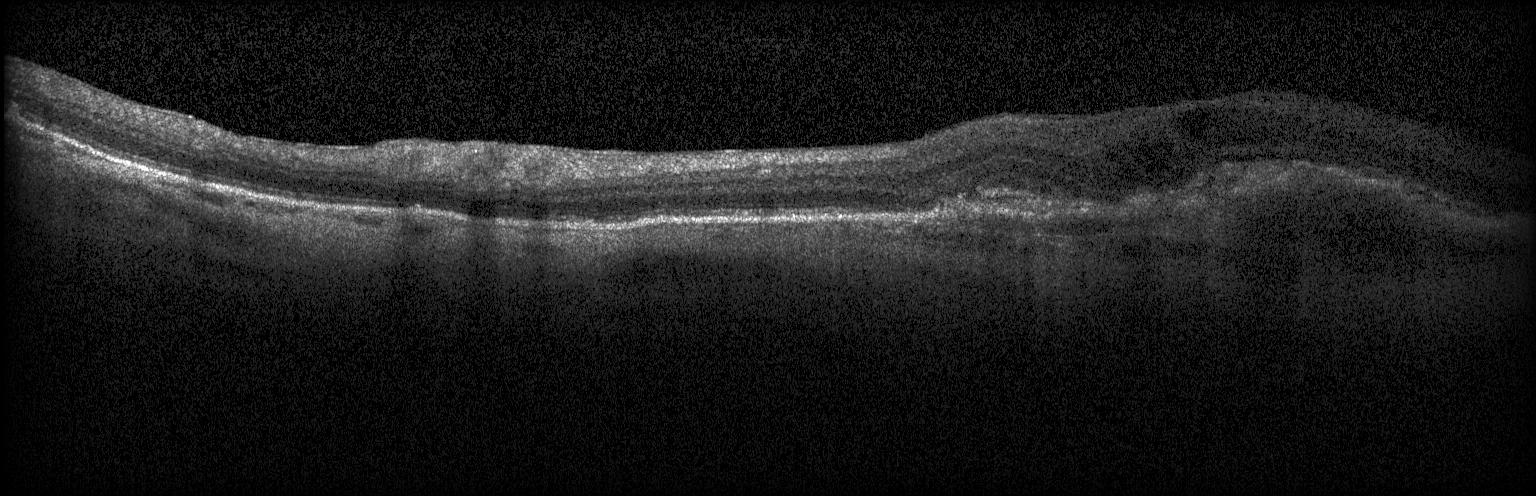 Retinal OCT B-scan — A choroidal neovascular membrane.